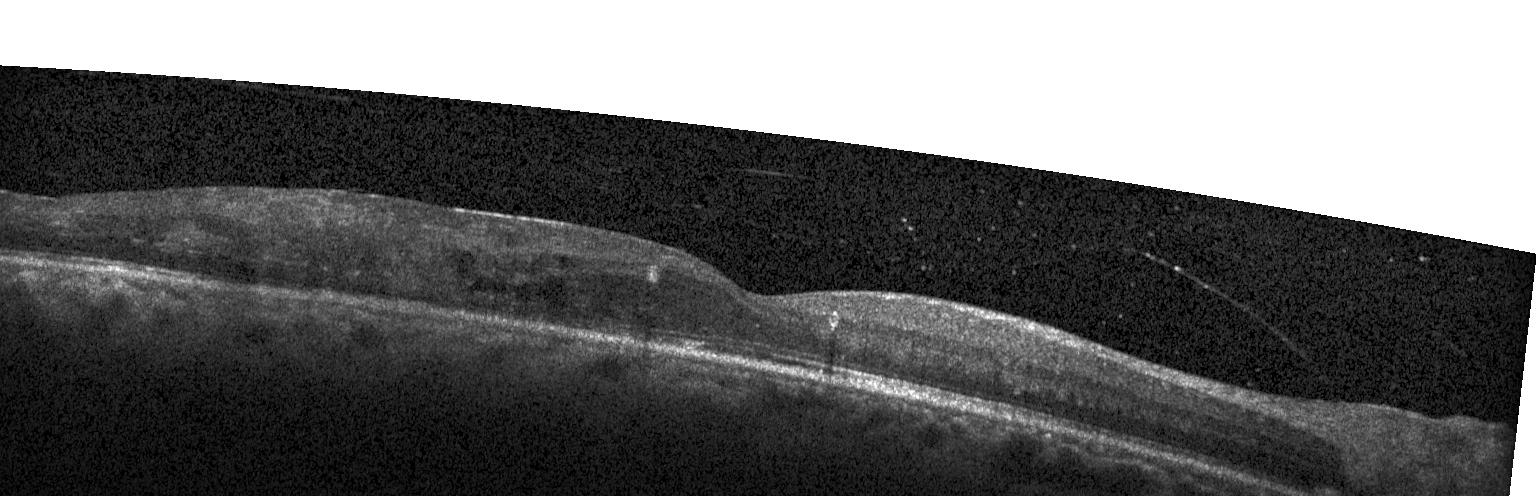 Retinal OCT B-scan · SD-OCT · Heidelberg Spectralis OCT system · through the macula.
The scan shows diabetic macular edema (DME).